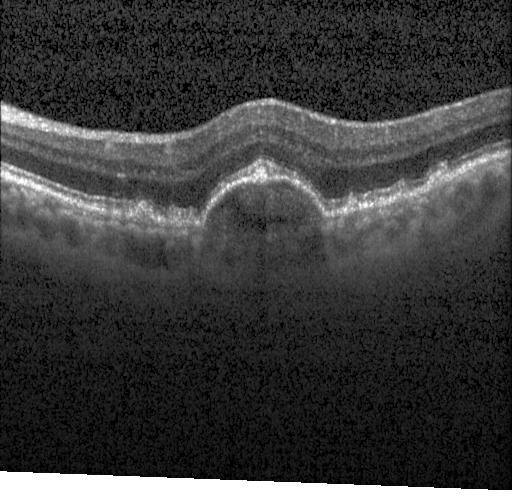
Optical coherence tomography scan. OCT finding: drusen.